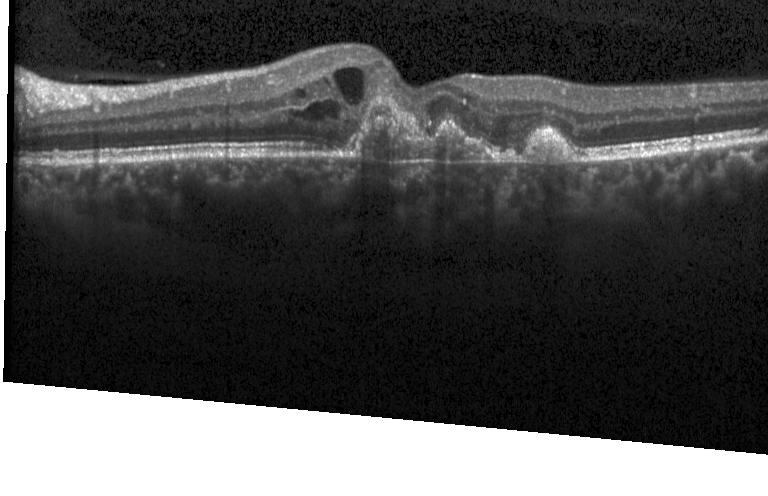 OCT finding: CNV.